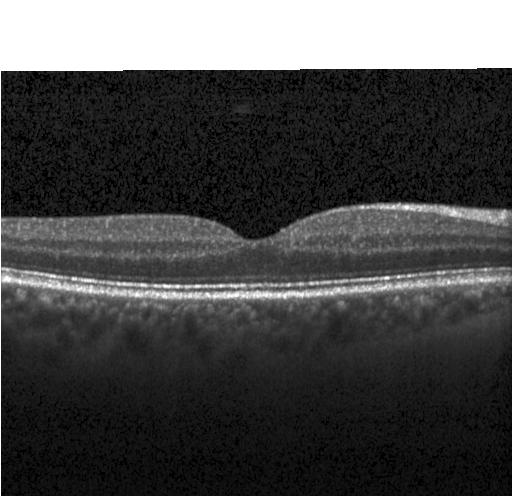

Acquired on a Heidelberg Spectralis; horizontal scan through the fovea; spectral-domain optical coherence tomography; optical coherence tomography B-scan. Dx: no evidence of CNV, DME, or drusen.